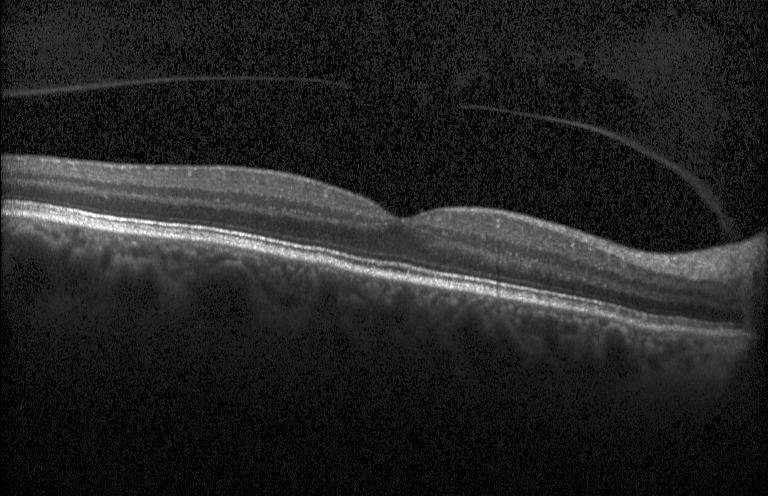
Impression: no choroidal neovascularization, diabetic macular edema, or drusen.